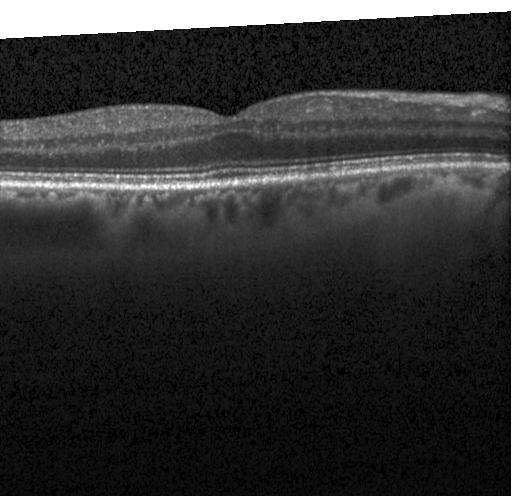 OCT line scan. Heidelberg Spectralis.
Diagnosis: no evidence of choroidal neovascularization, diabetic macular edema, or drusen.